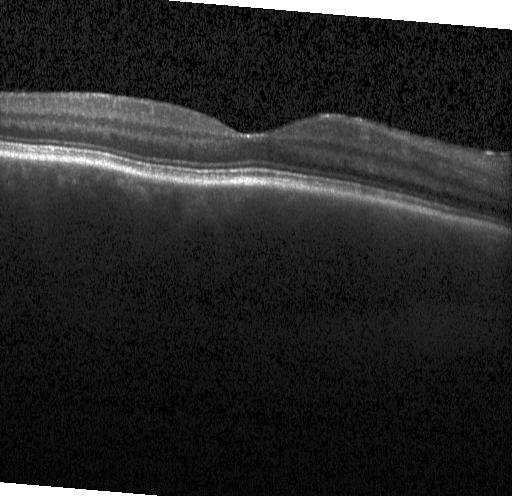
Optical coherence tomography B-scan — Finding: no evidence of choroidal neovascularization, diabetic macular edema, or drusen.